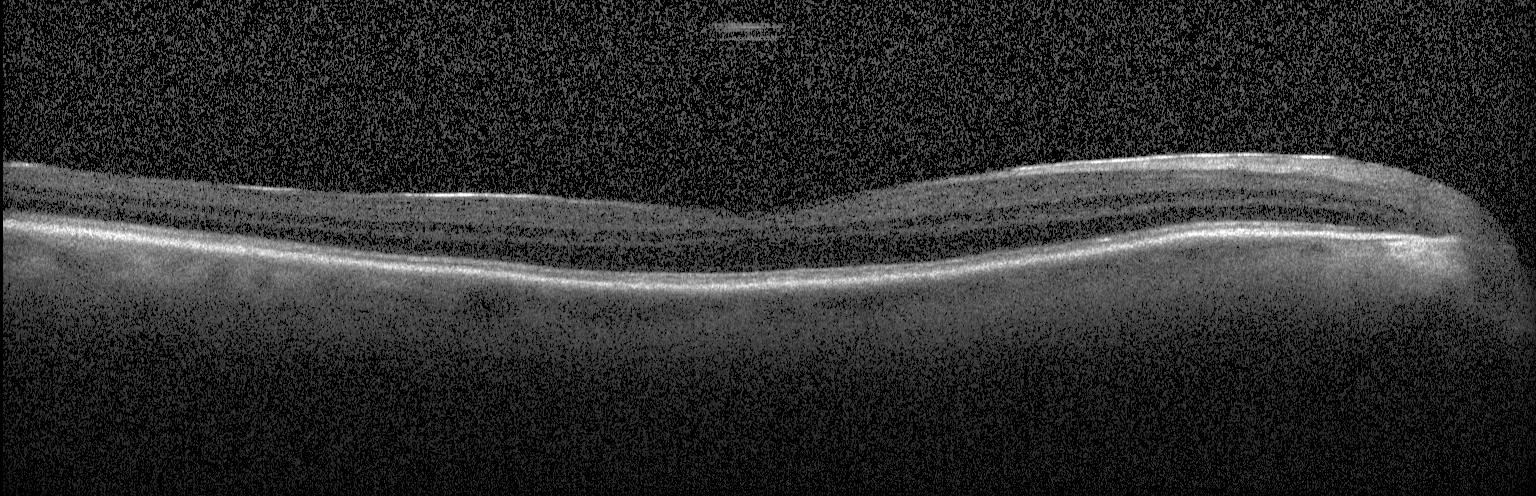 Spectral-domain OCT. OCT B-scan. No choroidal neovascularization, diabetic macular edema, or drusen.